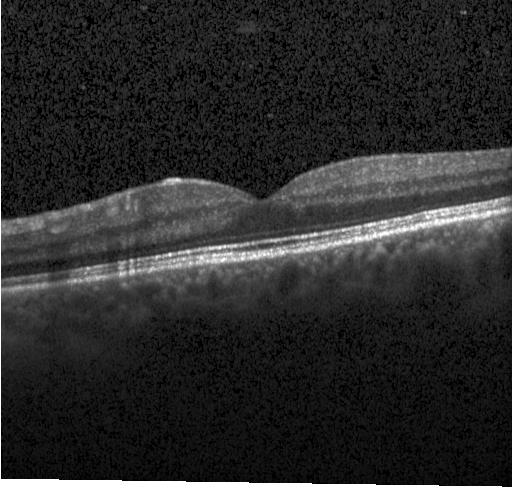 Impression: neither CNV, DME, nor drusen.